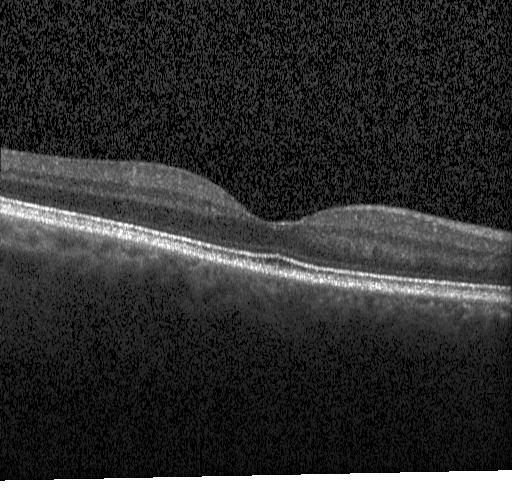
OCT B-scan. Diagnosis: no evidence of choroidal neovascularization, diabetic macular edema, or drusen.